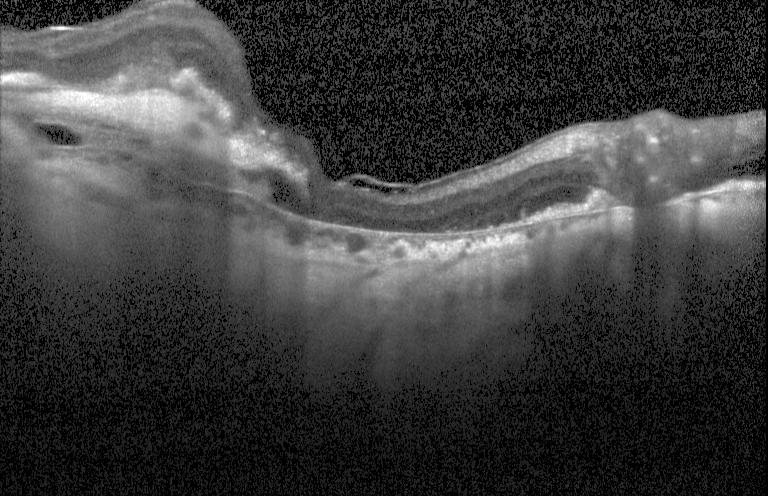 Spectral-domain OCT, macular scan, OCT line scan. Finding: a choroidal neovascular membrane.